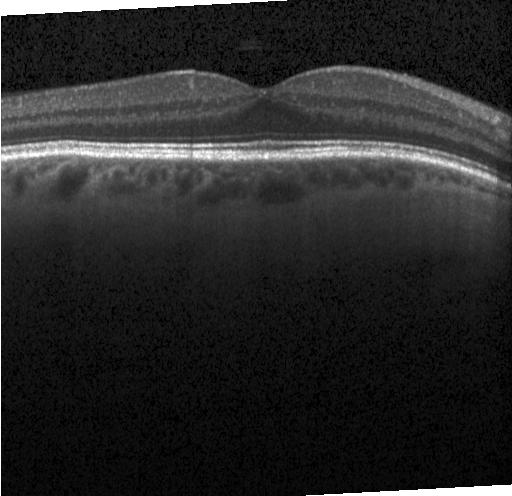

OCT B-scan; horizontal scan through the fovea; Heidelberg Spectralis; spectral-domain OCT
The scan shows no choroidal neovascularization, diabetic macular edema, or drusen.